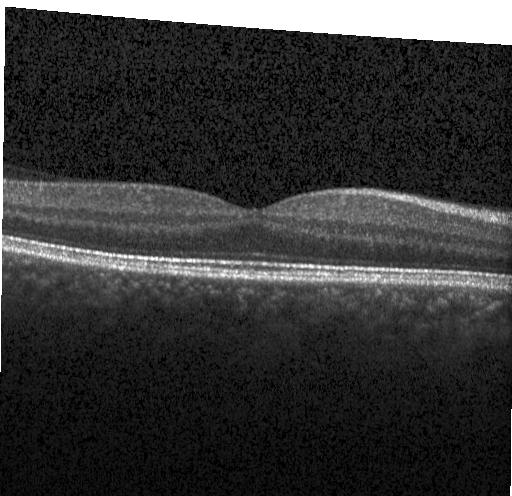 Macular scan · optical coherence tomography scan — The scan shows no evidence of choroidal neovascularization, diabetic macular edema, or drusen.